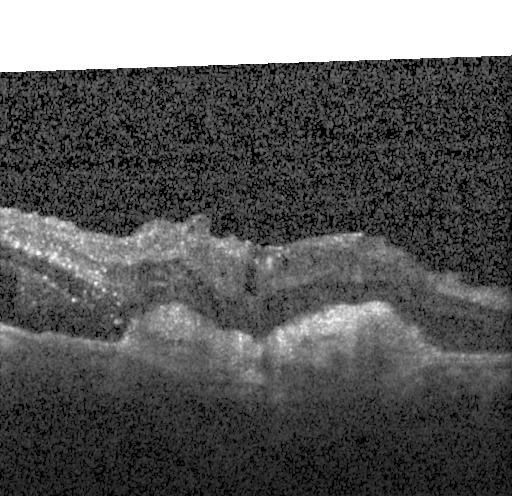

Optical coherence tomography B-scan · acquired on a Heidelberg Spectralis · spectral-domain OCT. Finding: choroidal neovascularization (CNV).